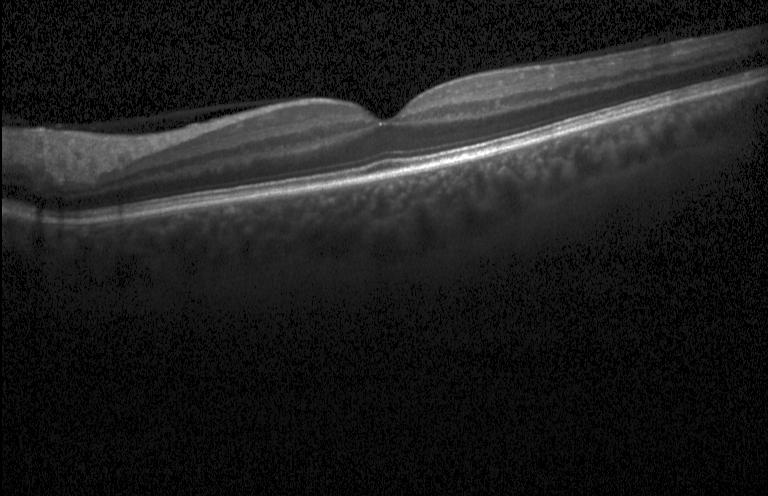

Diagnosis: no choroidal neovascularization, diabetic macular edema, or drusen.